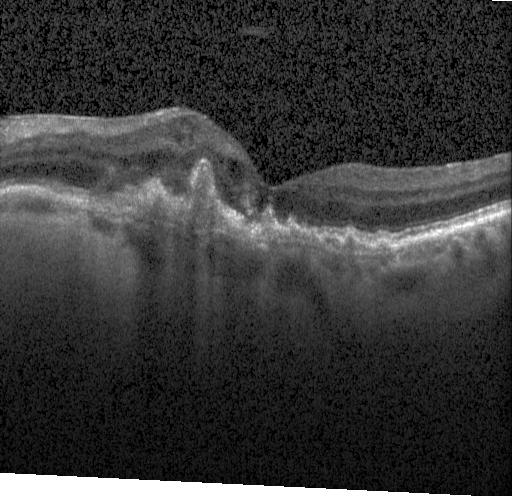
OCT scan showing choroidal neovascularization.